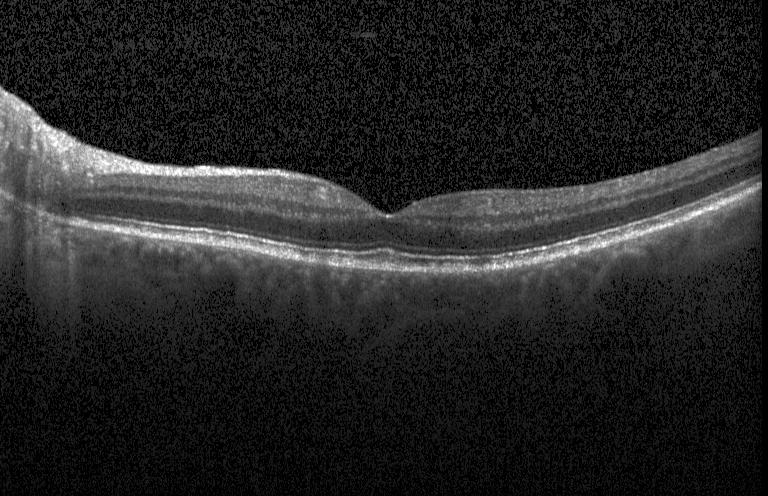
Retinal OCT B-scan. Instrument: Heidelberg Spectralis.
Assessment: neither choroidal neovascularization, diabetic macular edema, nor drusen.